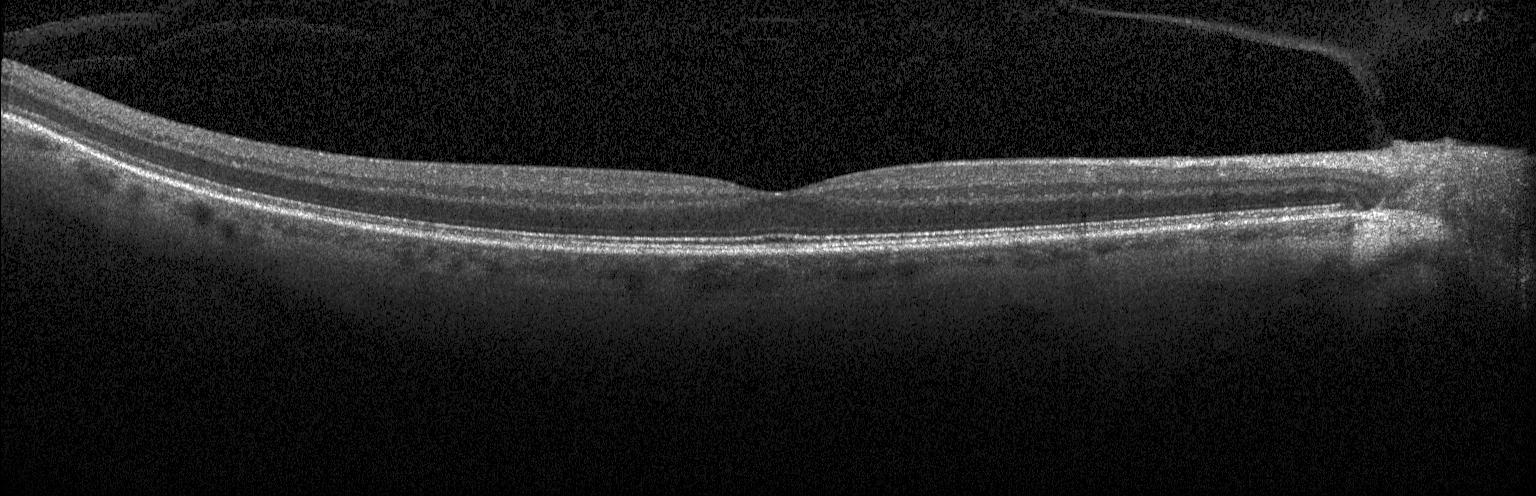 Retinal OCT B-scan — Dx: no choroidal neovascularization, no diabetic macular edema, and no drusen.